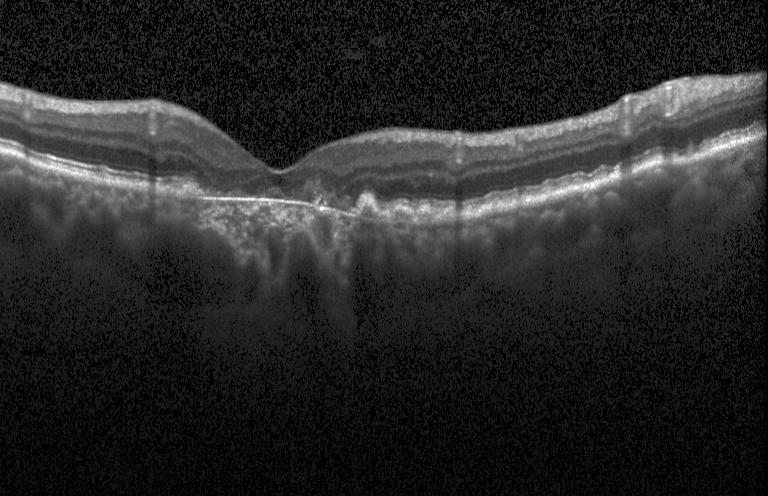
Retinal OCT cross-section showing a choroidal neovascular membrane.